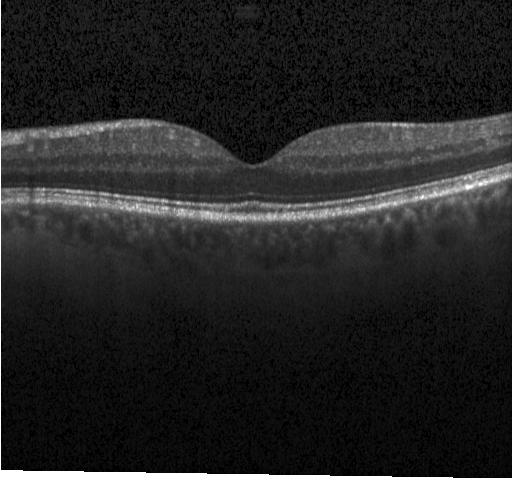
Finding: no CNV, no DME, and no drusen.